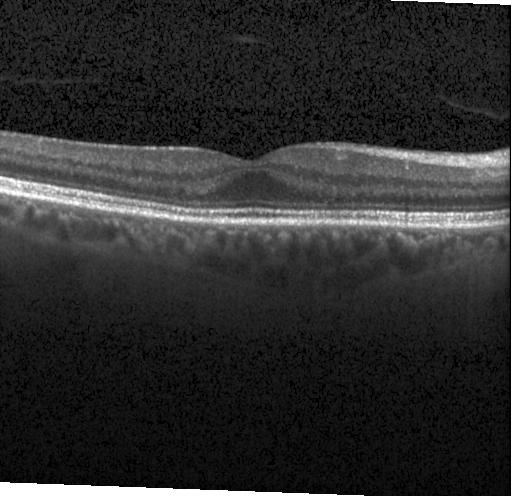 OCT line scan
Assessment: no evidence of choroidal neovascularization, diabetic macular edema, or drusen.